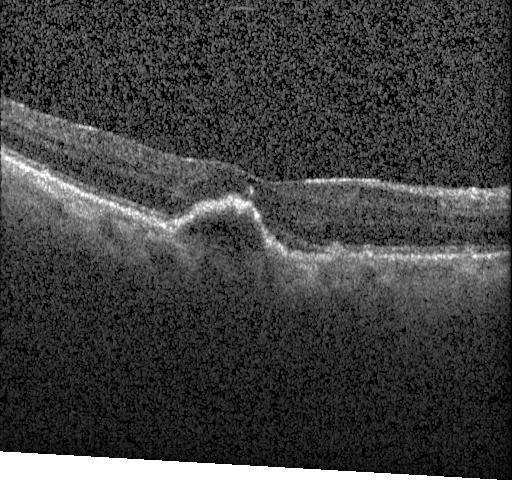 Finding: a choroidal neovascular membrane.